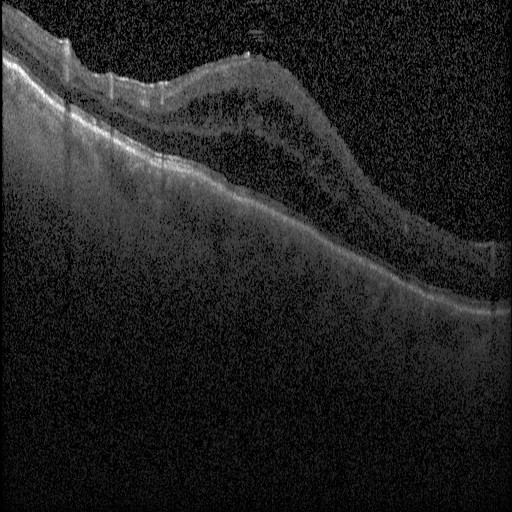
OCT B-scan showing diabetic macular edema (DME).